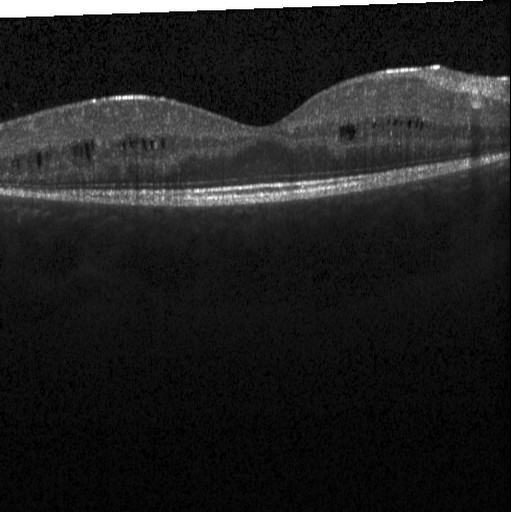
Spectral-domain OCT B-scan: DME.